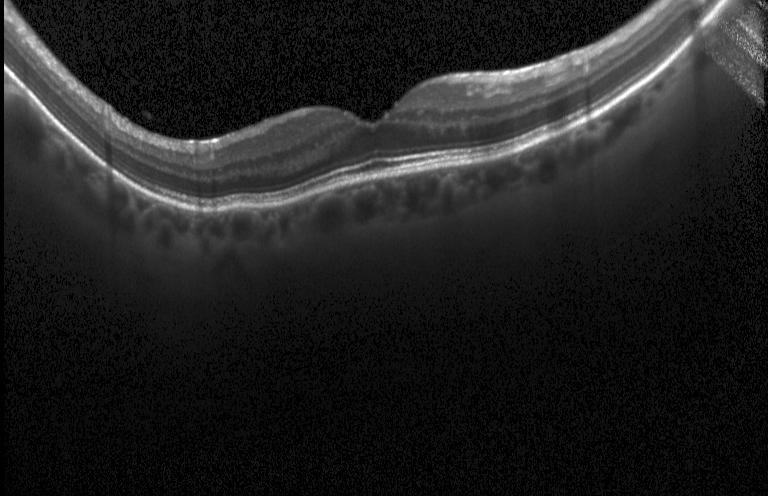 Optical coherence tomography scan — Impression: neither choroidal neovascularization, diabetic macular edema, nor drusen.